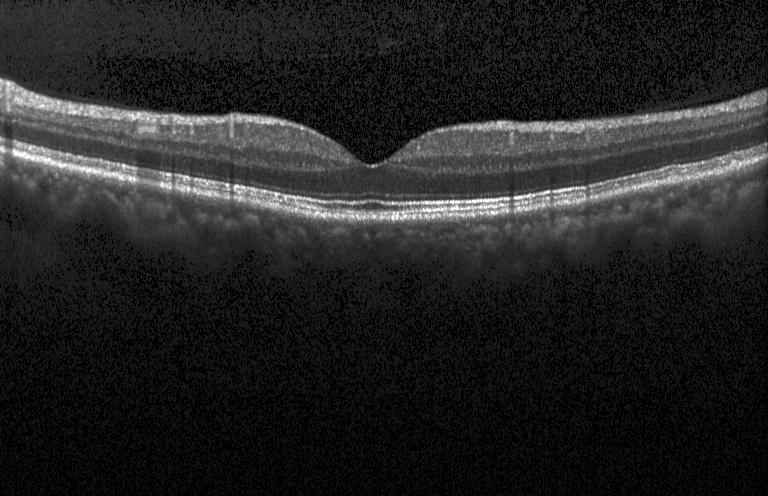
OCT B-scan. Macular scan. Heidelberg Spectralis OCT system. Spectral-domain optical coherence tomography
Finding: no choroidal neovascularization, no diabetic macular edema, and no drusen.